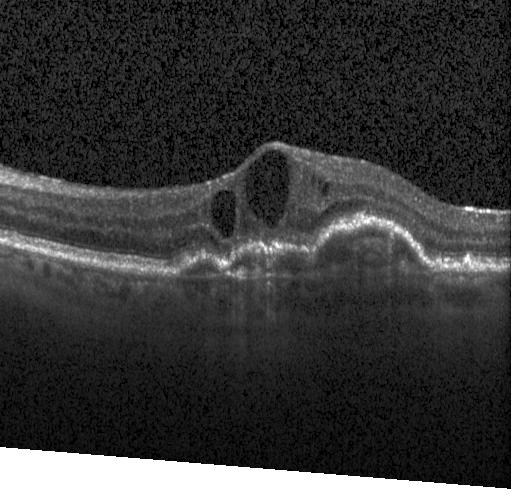 Optical coherence tomography scan · spectral-domain OCT.
The scan shows a choroidal neovascular membrane.